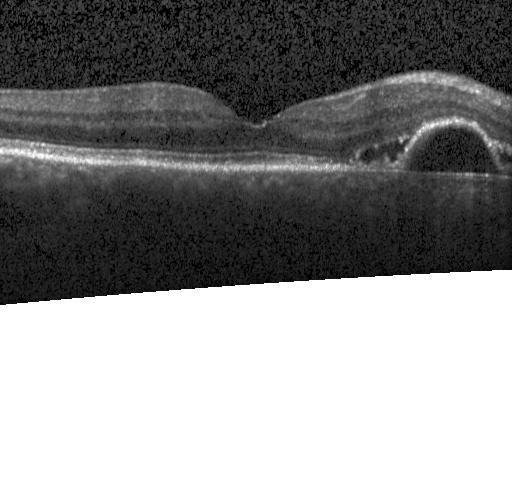
The scan shows a choroidal neovascular membrane.